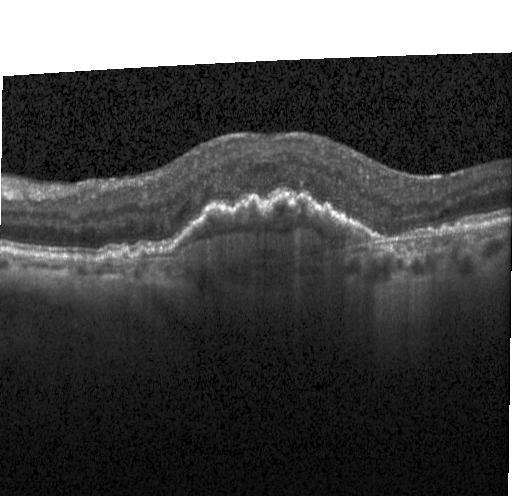 Finding: choroidal neovascularization (CNV).